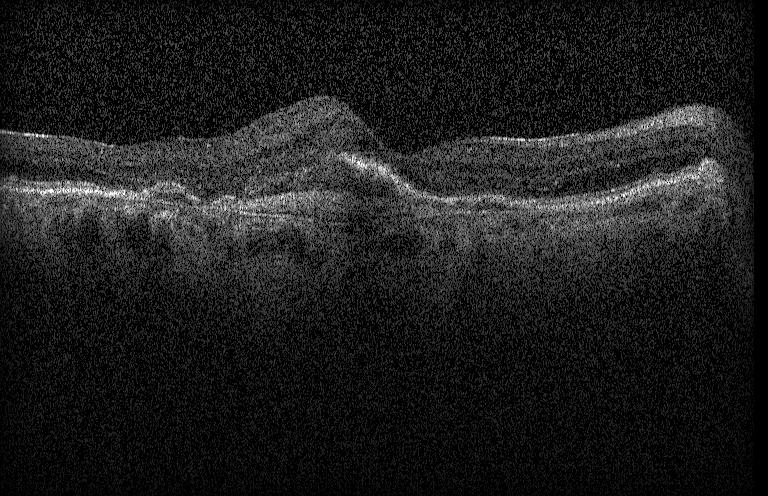

SD-OCT; optical coherence tomography B-scan; macular scan; Heidelberg Spectralis.
Choroidal neovascularization.